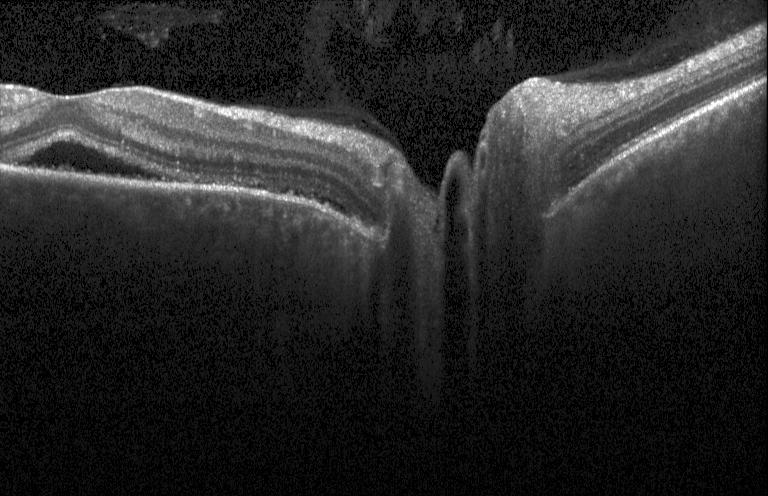 OCT finding: CNV.